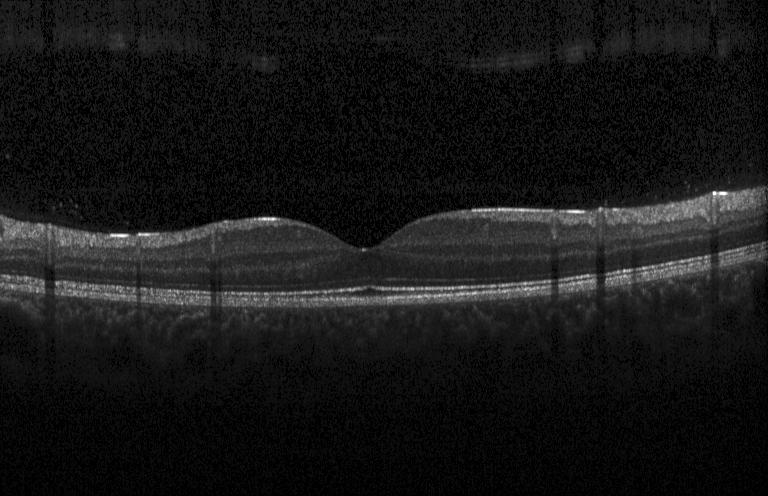 Assessment: neither choroidal neovascularization, diabetic macular edema, nor drusen.